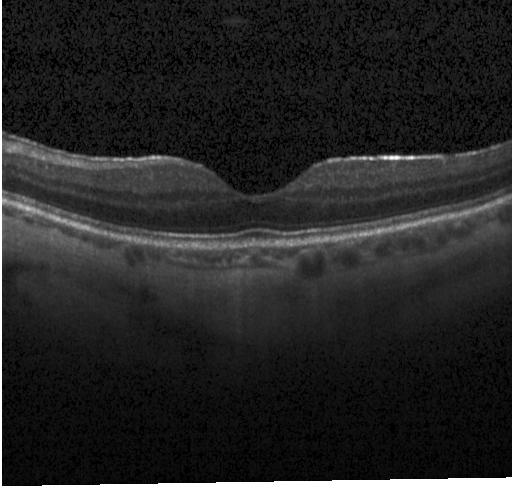
OCT finding: no choroidal neovascularization, no diabetic macular edema, and no drusen.